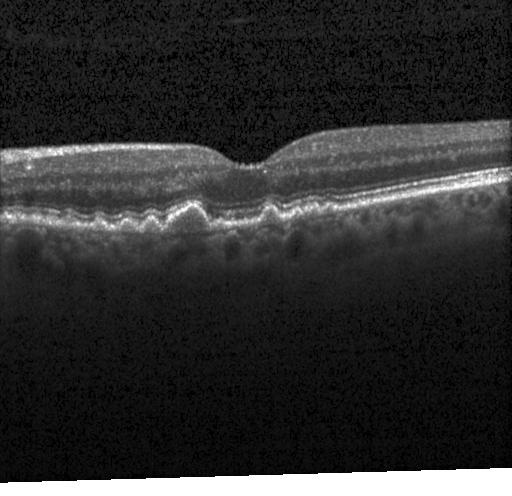 Retinal OCT B-scan, centered on the fovea, SD-OCT, Heidelberg Spectralis OCT system — Assessment: drusen.